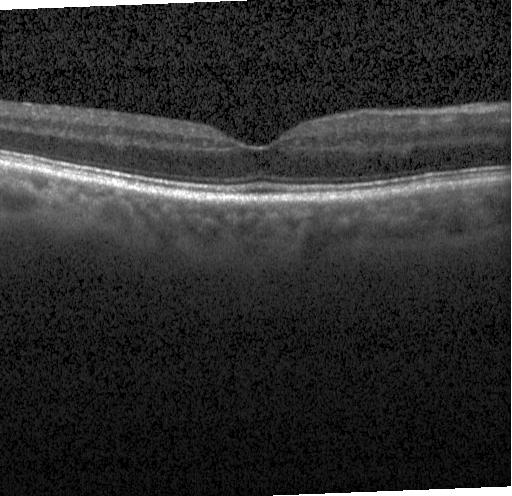

Retinal OCT cross-section showing no CNV, no DME, and no drusen.